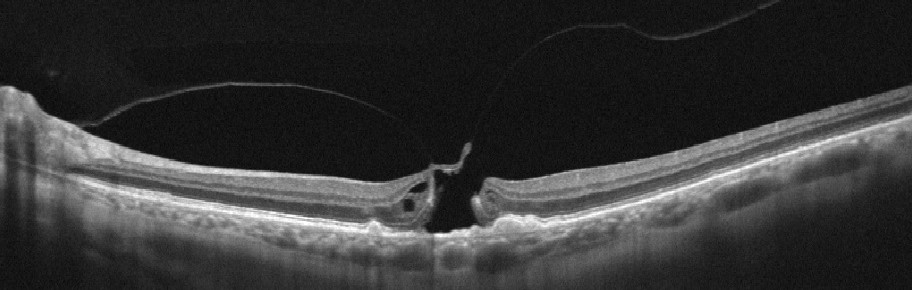

Instrument: Optovue Avanti RTVue XR. Fovea-centered. Optical coherence tomography scan. This B-scan demonstrates vitreomacular interface disease (VID).